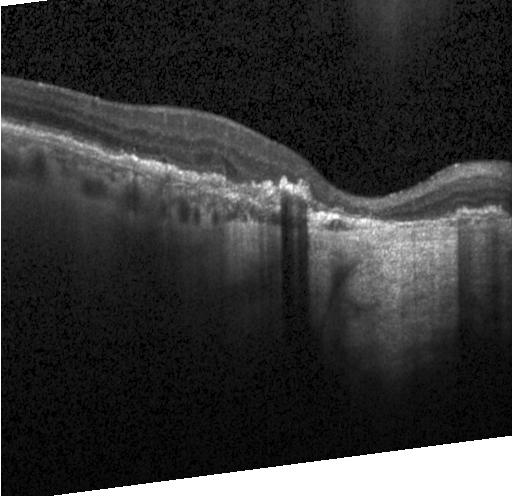

Optical coherence tomography B-scan. Heidelberg Spectralis OCT system. Finding: CNV.